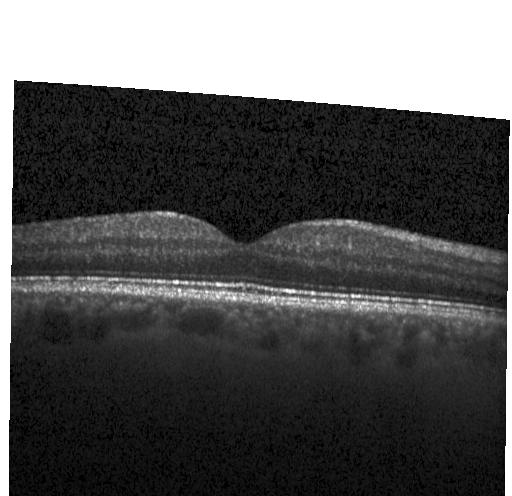

Optical coherence tomography B-scan · fovea-centered · Heidelberg Spectralis · spectral-domain optical coherence tomography — Finding: no evidence of choroidal neovascularization, diabetic macular edema, or drusen.